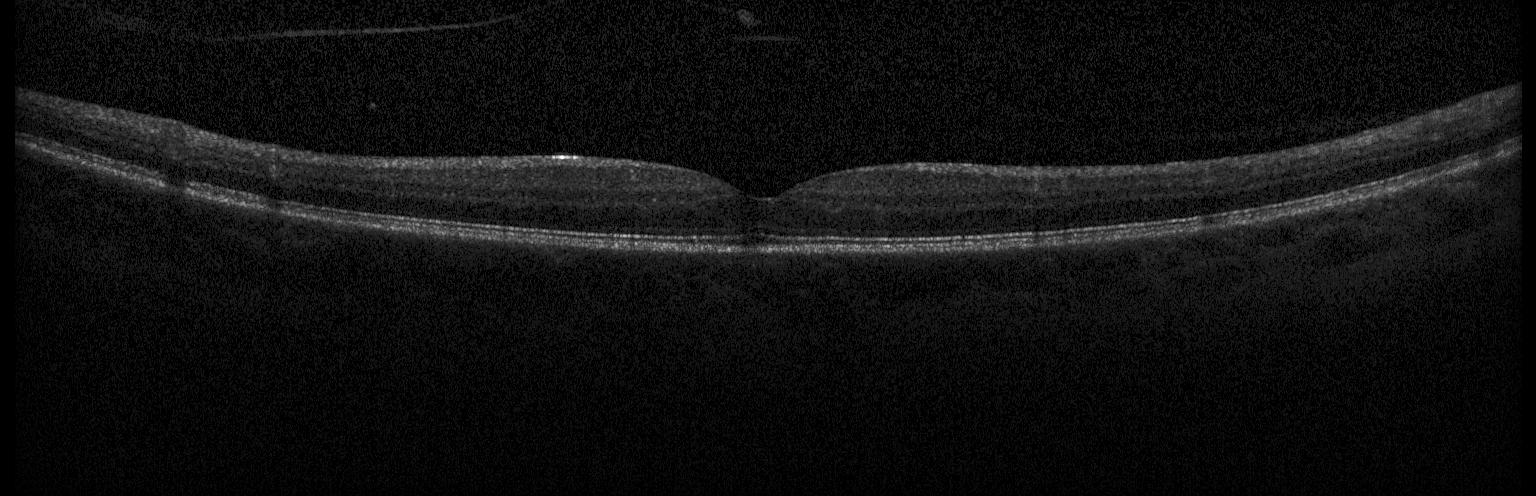
Optical coherence tomography B-scan
Diagnosis: no choroidal neovascularization, no diabetic macular edema, and no drusen.